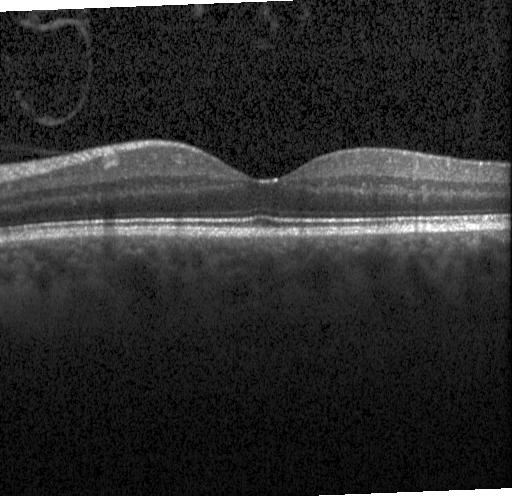
Spectral-domain OCT, optical coherence tomography B-scan. Impression: no evidence of choroidal neovascularization, diabetic macular edema, or drusen.